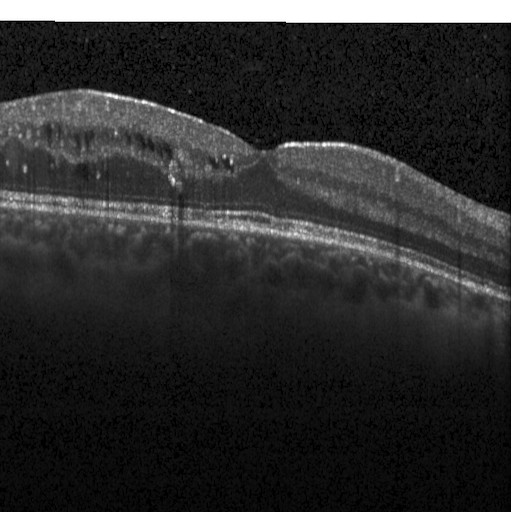
SD-OCT. Optical coherence tomography scan. Centered on the fovea
The scan shows diabetic macular edema.